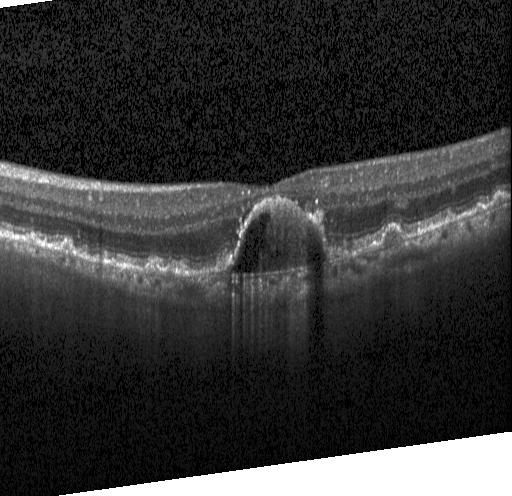

Through the macula · retinal OCT cross-section.
CNV.